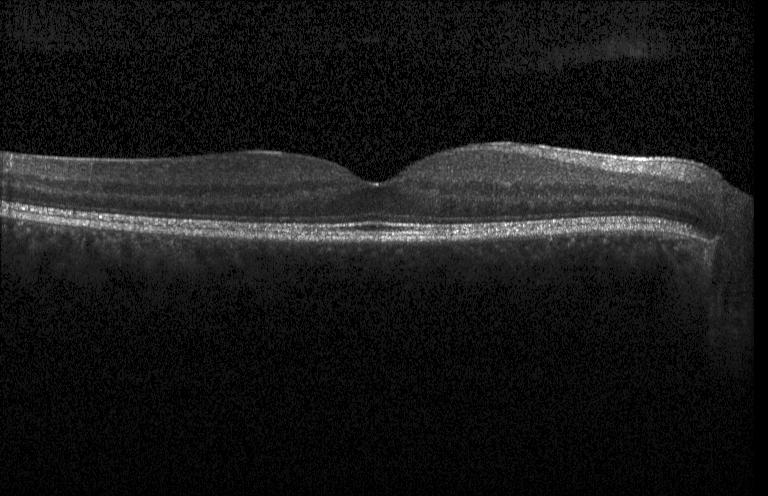

Macular OCT: neither choroidal neovascularization, diabetic macular edema, nor drusen.